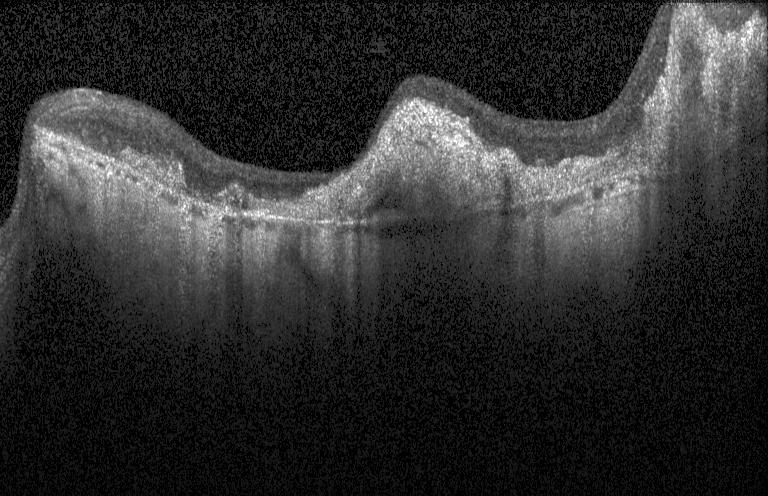 Retinal OCT cross-section. Finding: a choroidal neovascular membrane.